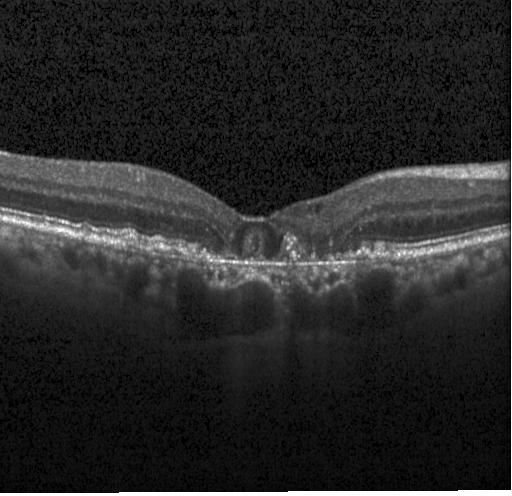 Macular OCT: a choroidal neovascular membrane.